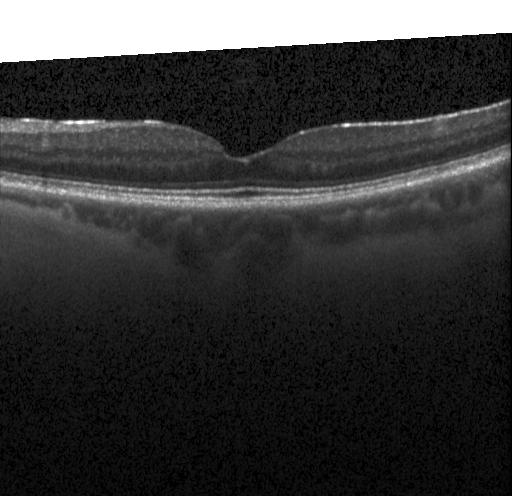

Macular OCT demonstrating no CNV, no DME, and no drusen.